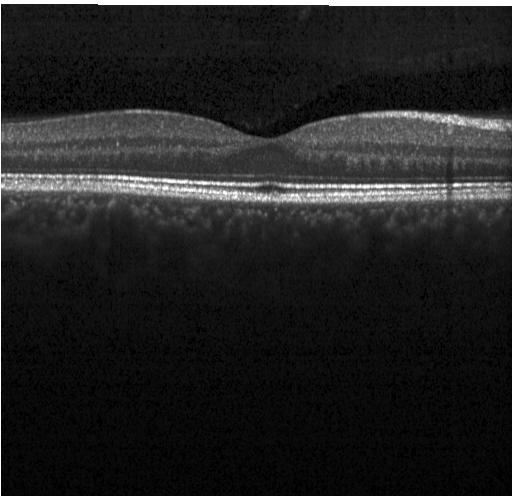 OCT B-scan. SD-OCT. Acquired on a Heidelberg Spectralis. Centered on the fovea. Impression: neither CNV, DME, nor drusen.